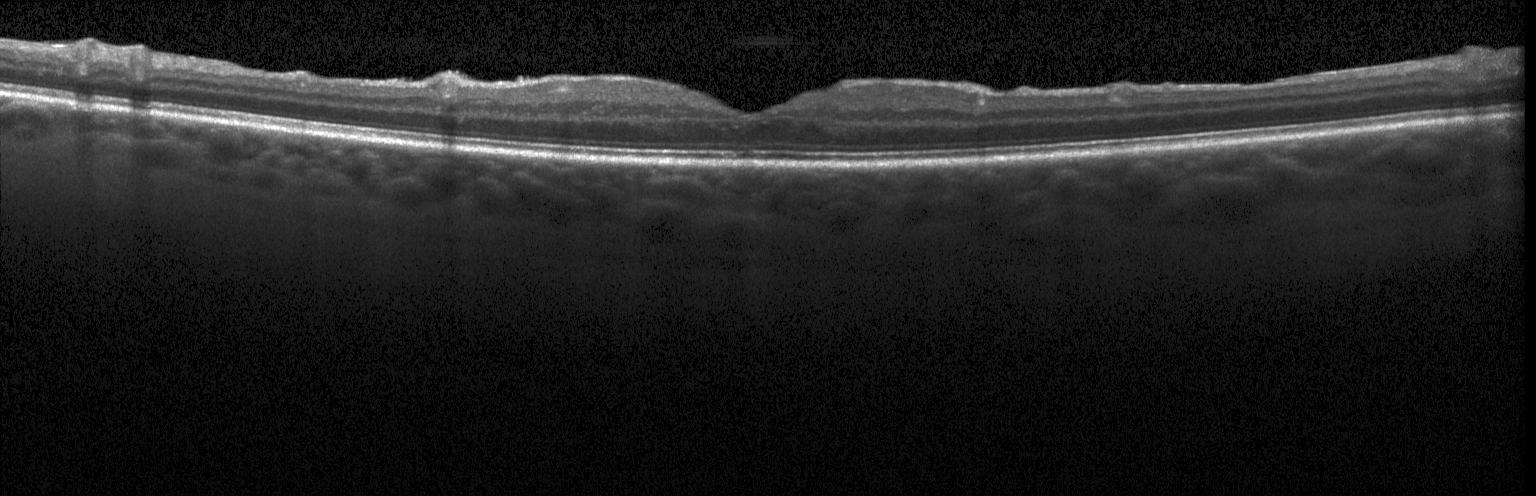 Retinal OCT cross-section.
Diagnosis: no choroidal neovascularization, no diabetic macular edema, and no drusen.